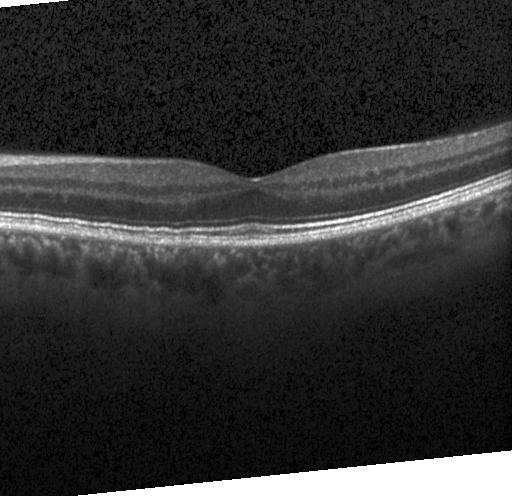
The scan shows neither CNV, DME, nor drusen.